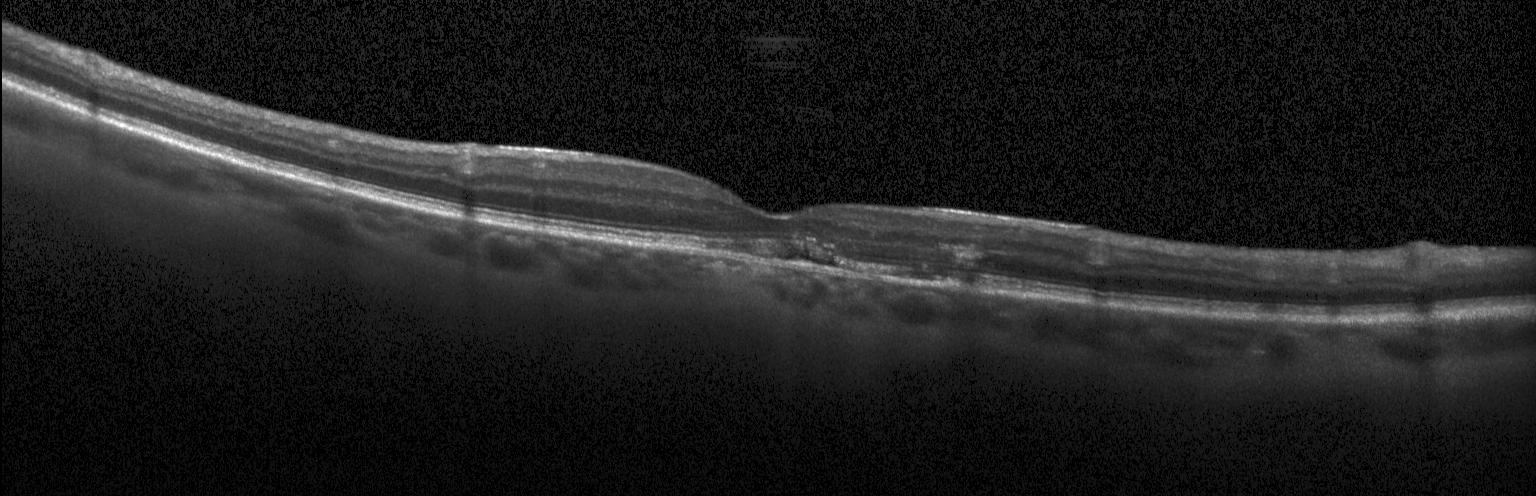
Fovea-centered, OCT line scan.
Assessment: CNV.